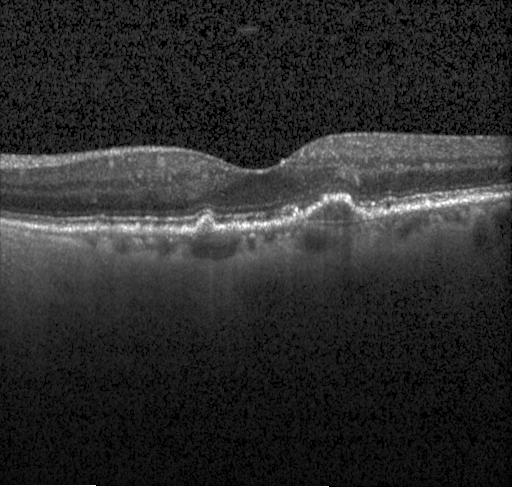 Acquired on a Heidelberg Spectralis. Centered on the fovea. Spectral-domain optical coherence tomography. Optical coherence tomography scan. This B-scan demonstrates drusen.